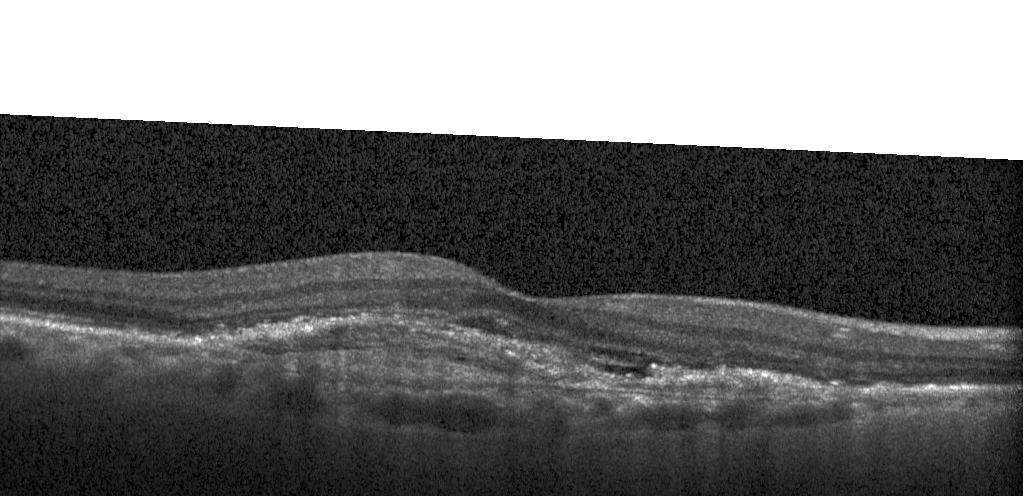

Diagnosis: choroidal neovascularization.